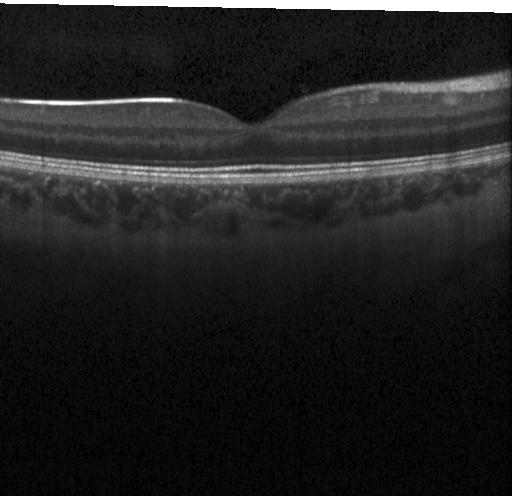
OCT scan showing no choroidal neovascularization, diabetic macular edema, or drusen.